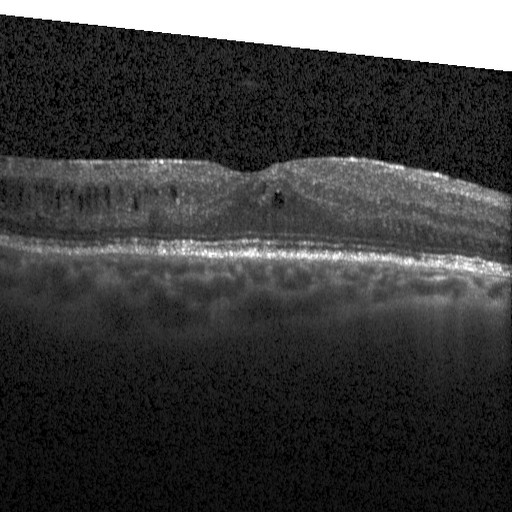
OCT line scan; spectral-domain OCT; Heidelberg Spectralis. This B-scan demonstrates diabetic macular edema (DME).